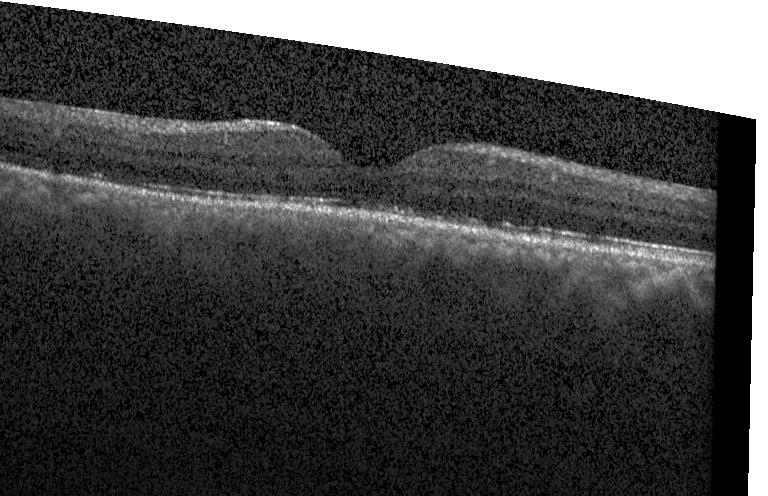

Impression: neither CNV, DME, nor drusen.